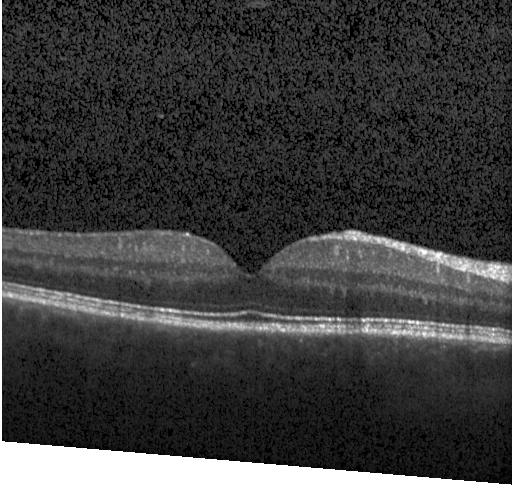 Spectral-domain optical coherence tomography · through the macula · Heidelberg Spectralis OCT system · optical coherence tomography B-scan
Finding: no evidence of choroidal neovascularization, diabetic macular edema, or drusen.